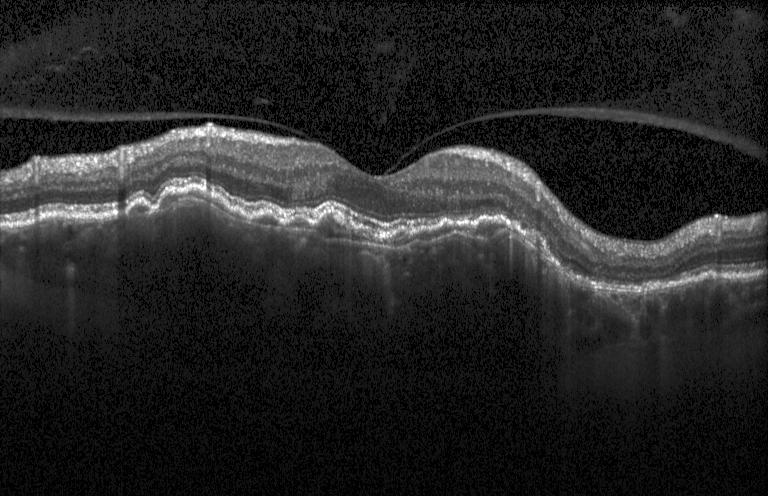
OCT B-scan.
Dx: CNV.